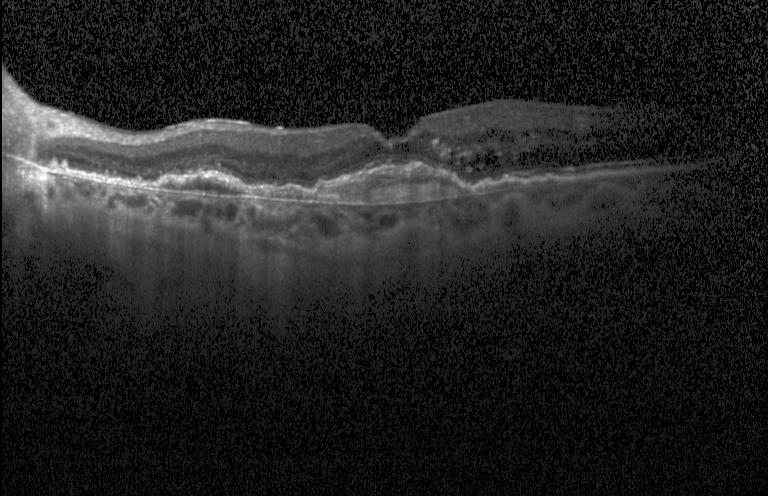
OCT B-scan. The scan shows CNV.